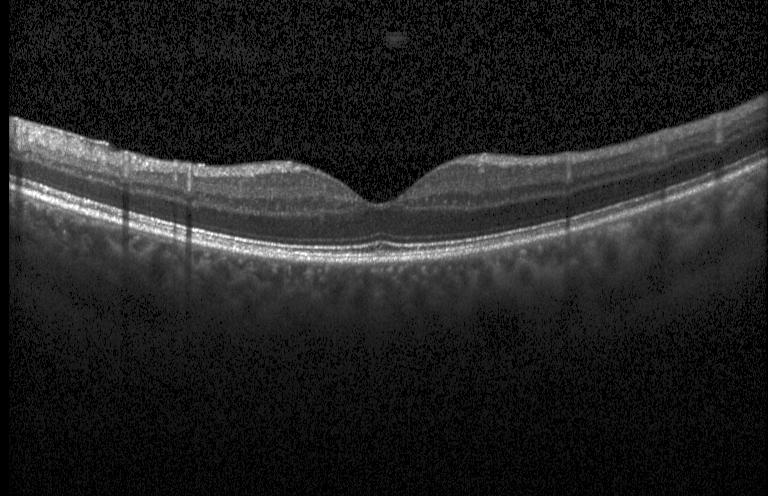
Centered on the fovea · retinal OCT cross-section.
The scan shows no evidence of choroidal neovascularization, diabetic macular edema, or drusen.